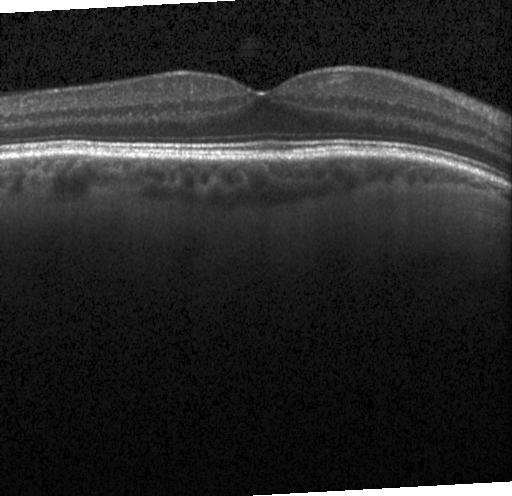
Optical coherence tomography B-scan. SD-OCT
This B-scan demonstrates no CNV, no DME, and no drusen.